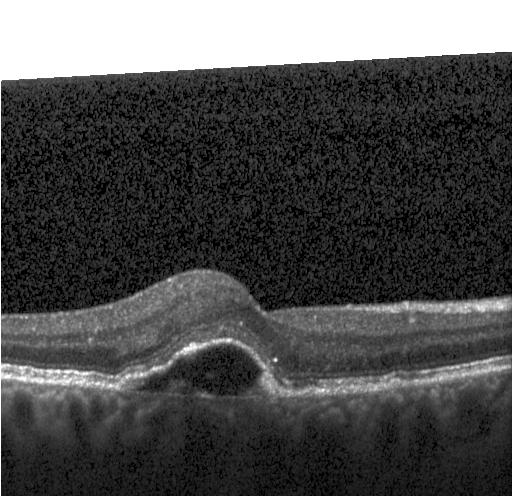 Instrument: Heidelberg Spectralis; OCT line scan; horizontal scan through the fovea.
Assessment: choroidal neovascularization.